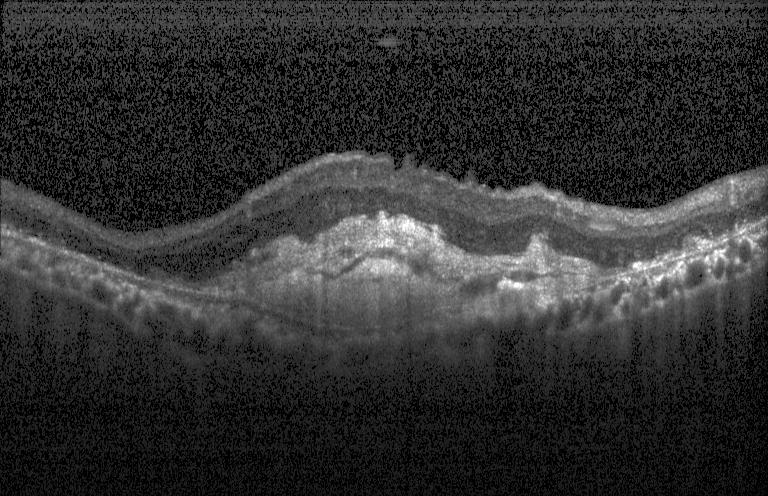

OCT line scan.
Impression: choroidal neovascularization.